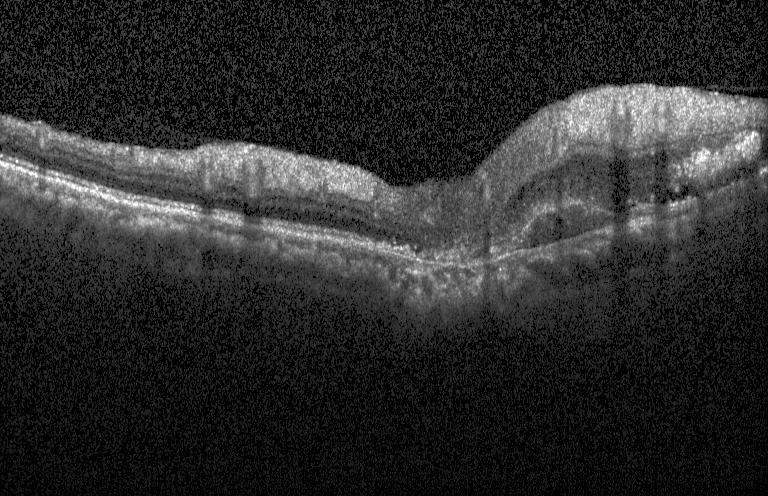 Dx: a choroidal neovascular membrane.